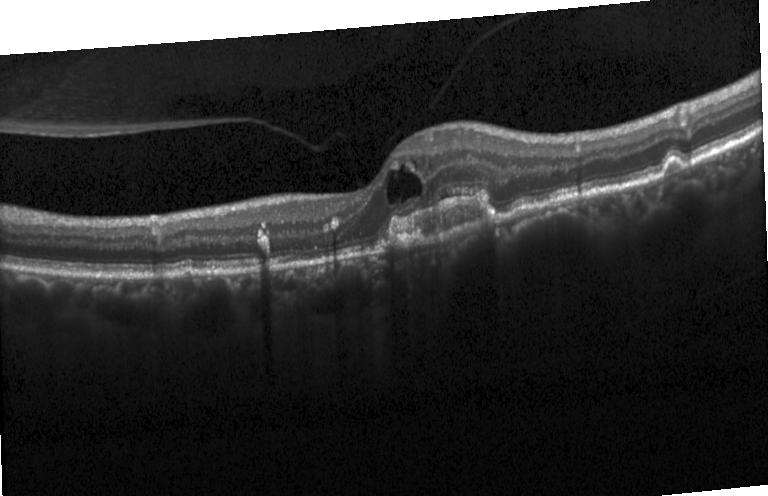 Spectral-domain optical coherence tomography; optical coherence tomography B-scan — OCT finding: CNV.